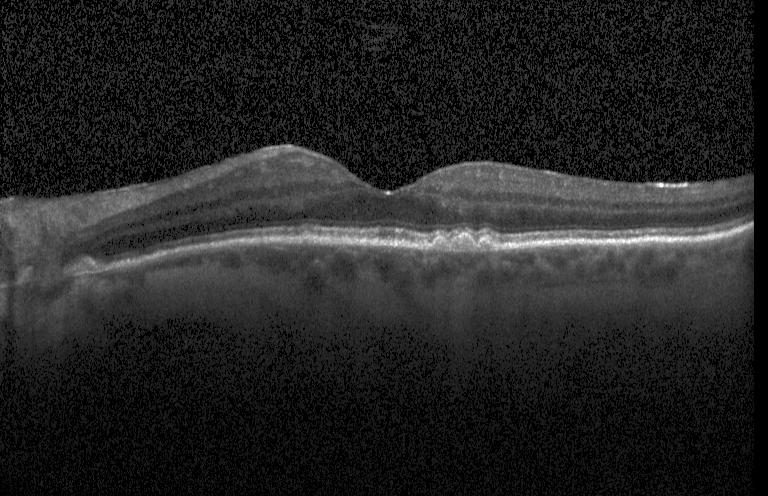 Retinal OCT cross-section, spectral-domain OCT — Sub-RPE drusenoid deposits.